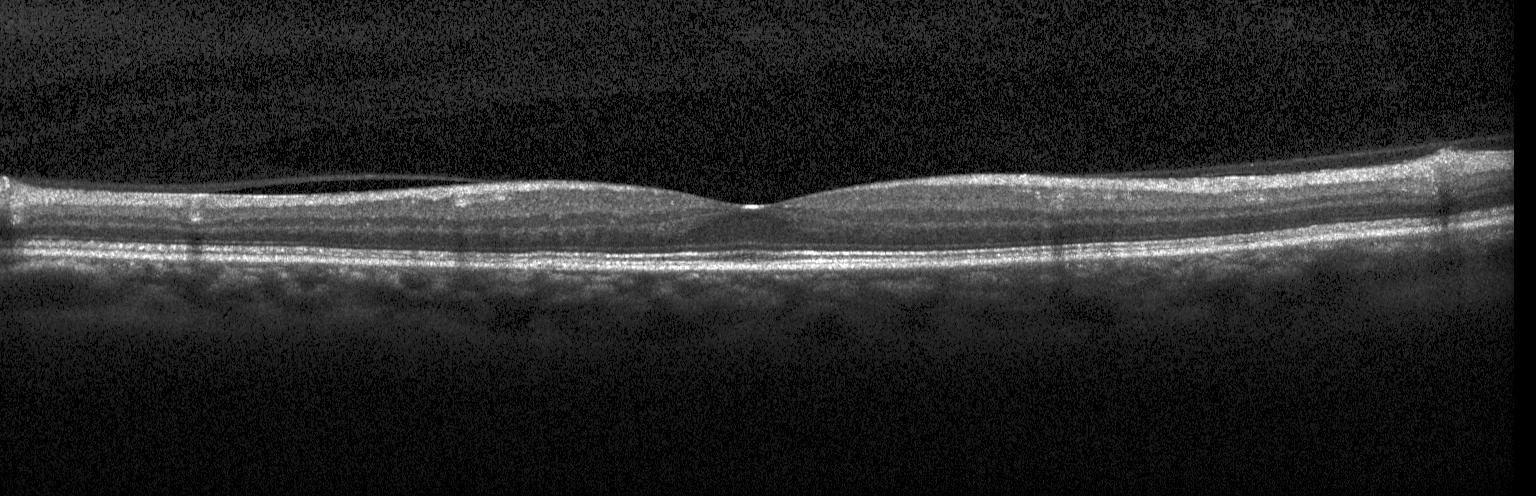
Heidelberg Spectralis · OCT B-scan · SD-OCT · horizontal scan through the fovea — Finding: neither choroidal neovascularization, diabetic macular edema, nor drusen.